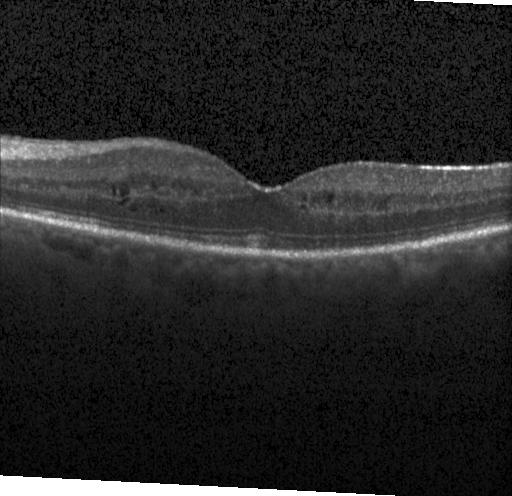 Assessment: diabetic macular edema (DME).